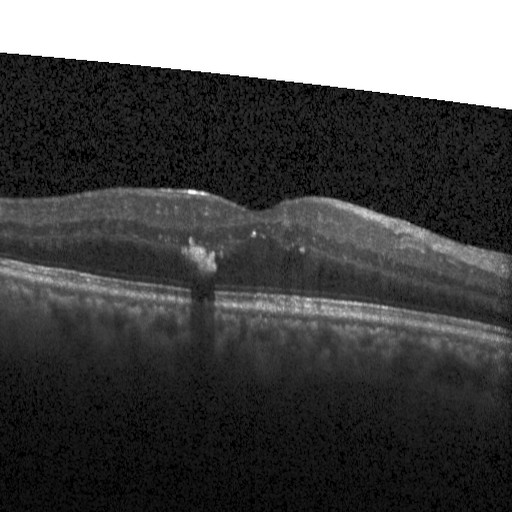

Retinal OCT cross-section.
Impression: diabetic macular edema.